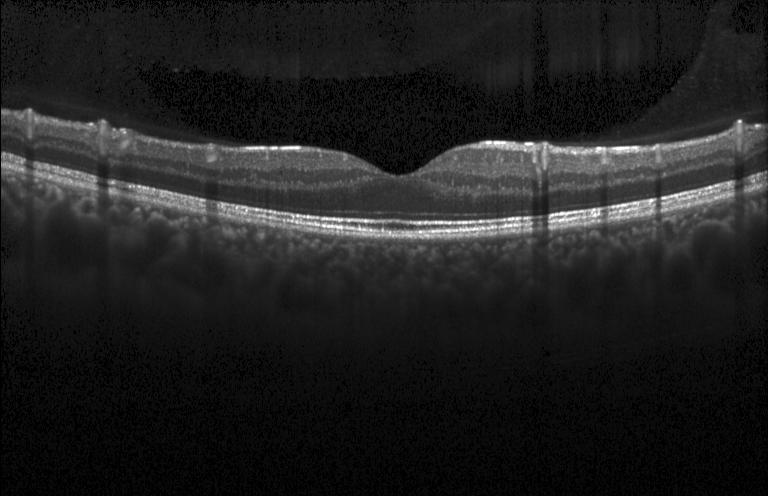

No CNV, no DME, and no drusen.